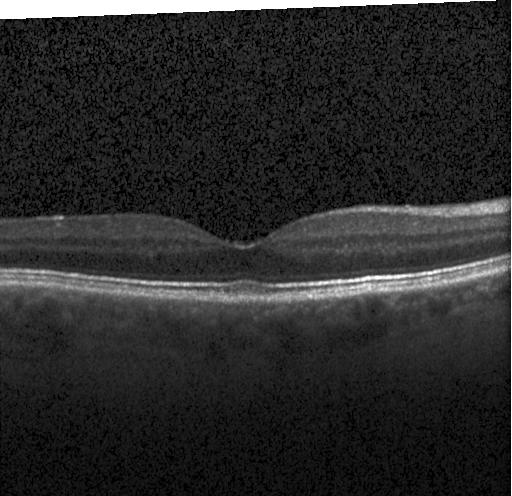 OCT B-scan showing no evidence of choroidal neovascularization, diabetic macular edema, or drusen.